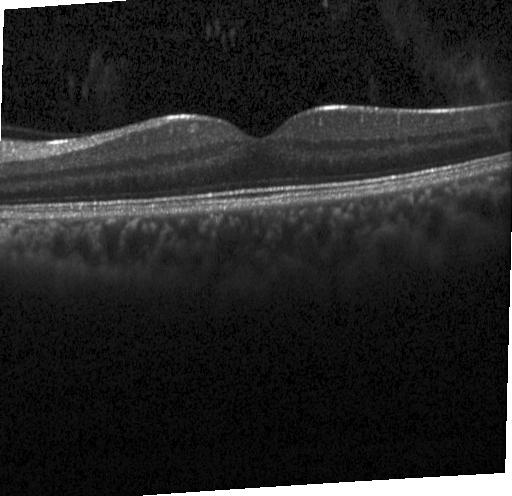 Optical coherence tomography scan. Macular scan. Diagnosis: no choroidal neovascularization, diabetic macular edema, or drusen.